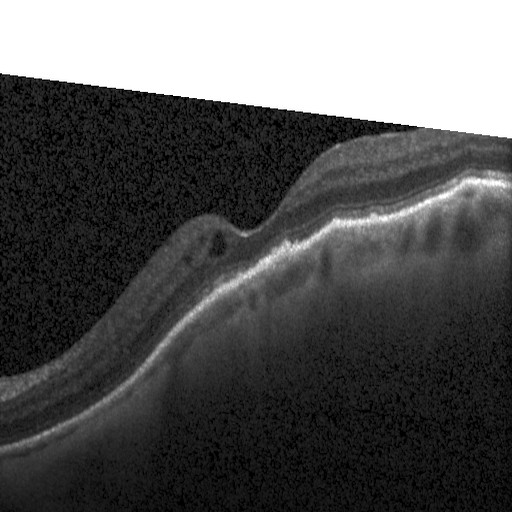

Macular OCT demonstrating diabetic macular edema (DME).